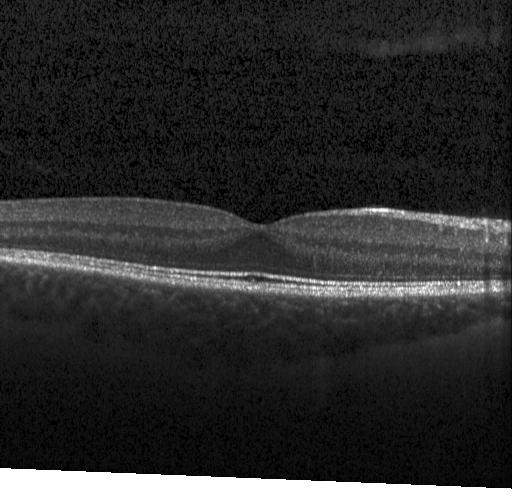

Optical coherence tomography B-scan
Assessment: no CNV, no DME, and no drusen.